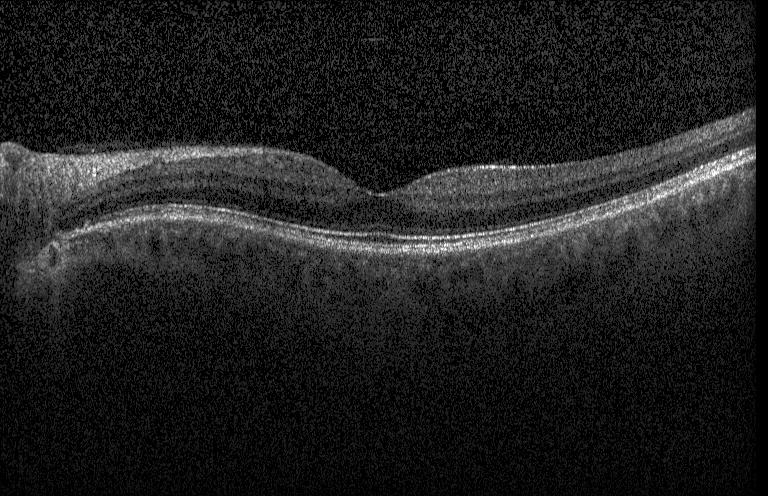 Through the macula, spectral-domain OCT, OCT B-scan.
OCT finding: no CNV, DME, or drusen.